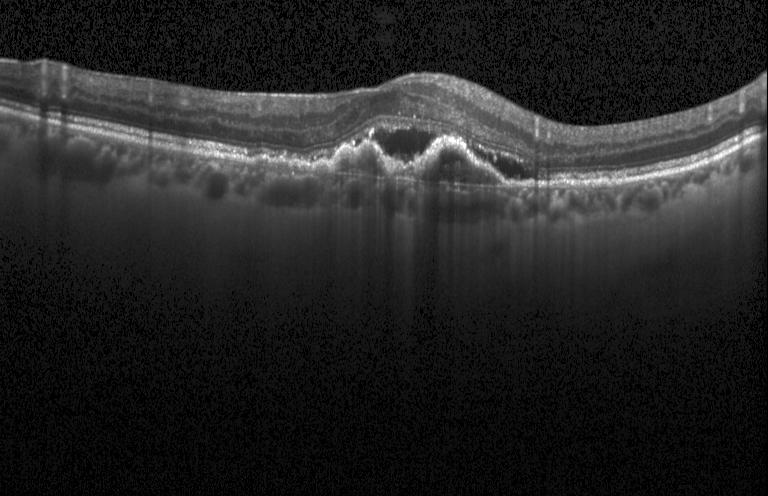 Impression: CNV.